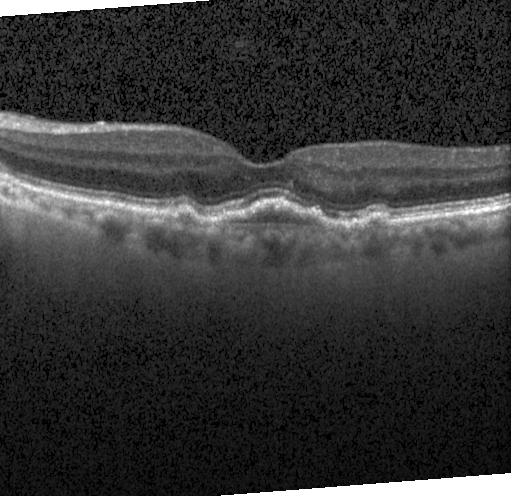 Spectral-domain OCT. Retinal OCT cross-section — Finding: CNV.